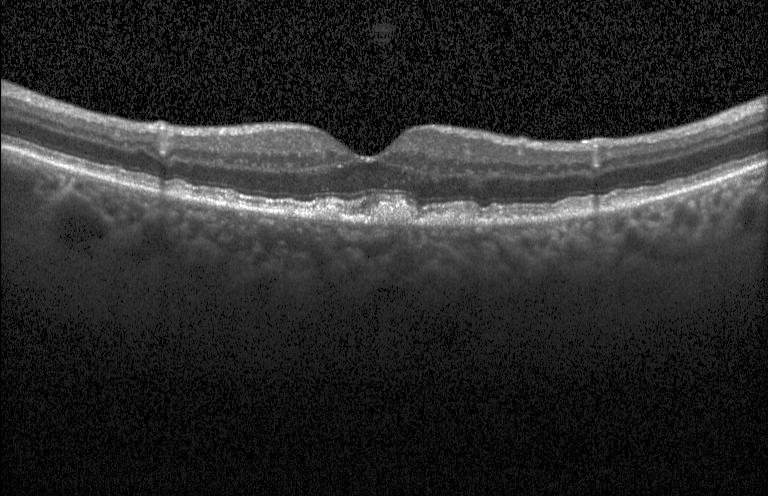
Optical coherence tomography scan.
Finding: a choroidal neovascular membrane.